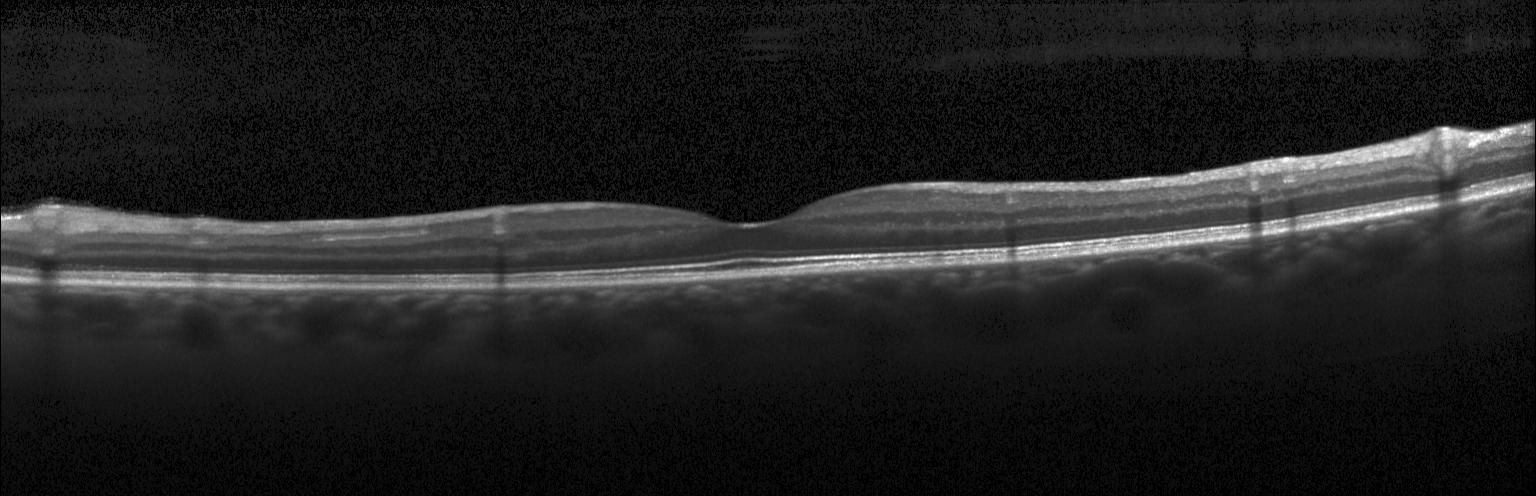 Finding: no choroidal neovascularization, diabetic macular edema, or drusen.